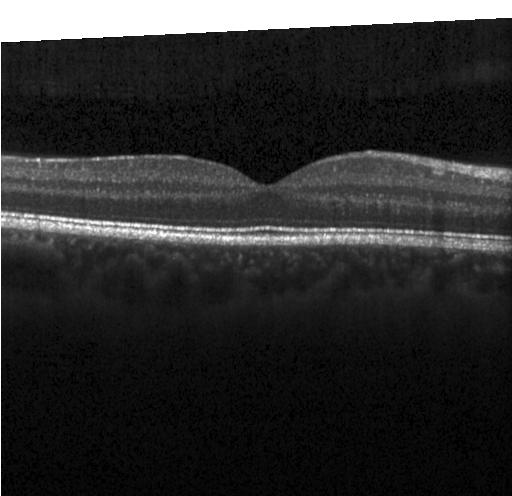 Spectral-domain OCT, fovea-centered, optical coherence tomography scan.
No evidence of choroidal neovascularization, diabetic macular edema, or drusen.